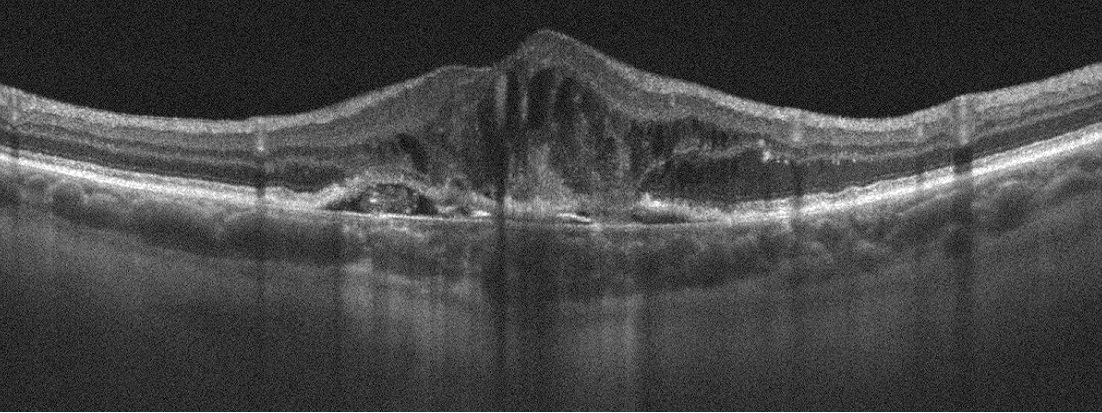 Optovue Avanti RTVue XR; retinal OCT cross-section — Impression: age-related macular degeneration.